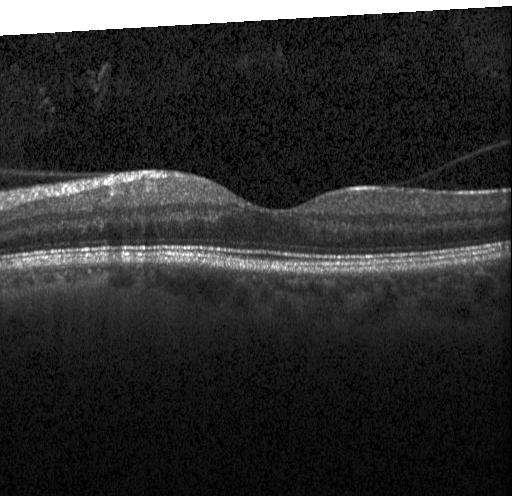 Retinal OCT cross-section showing no evidence of CNV, DME, or drusen.